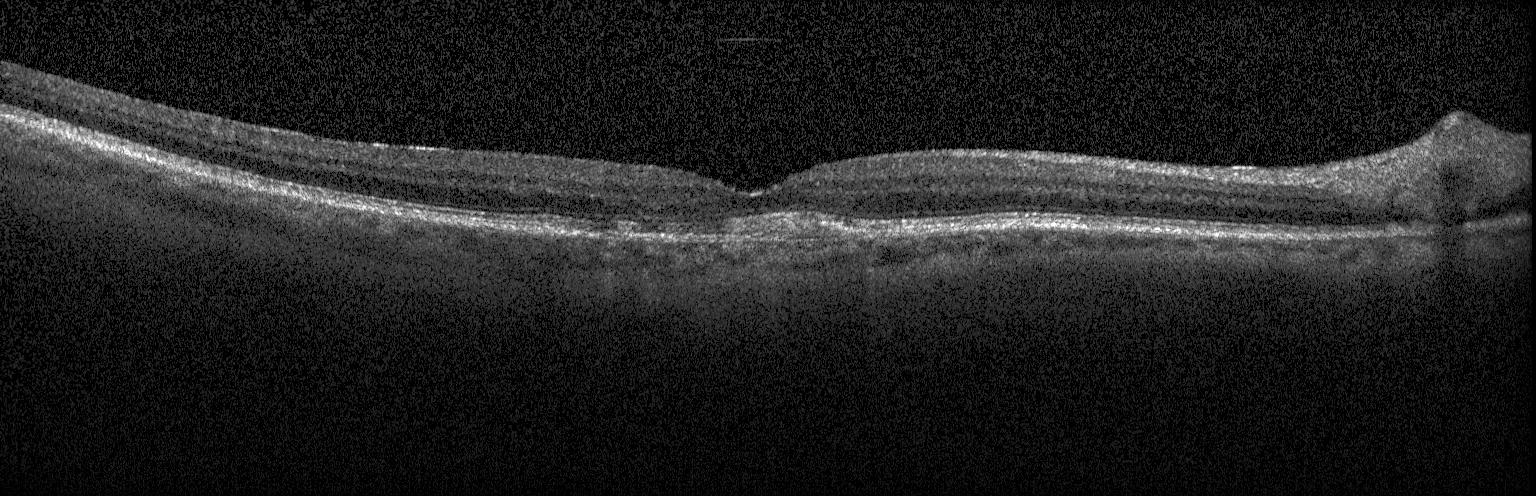 Macular OCT: CNV.